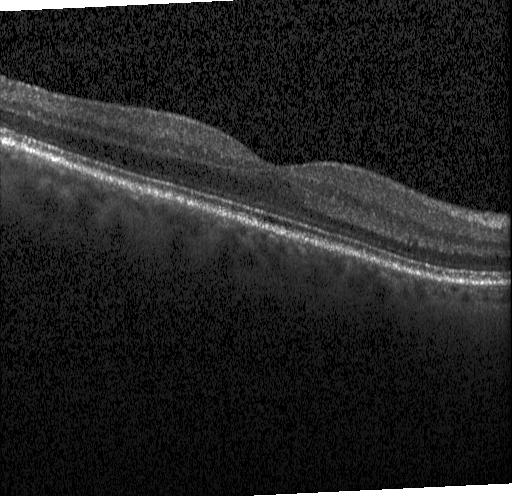
OCT finding: no choroidal neovascularization, diabetic macular edema, or drusen.